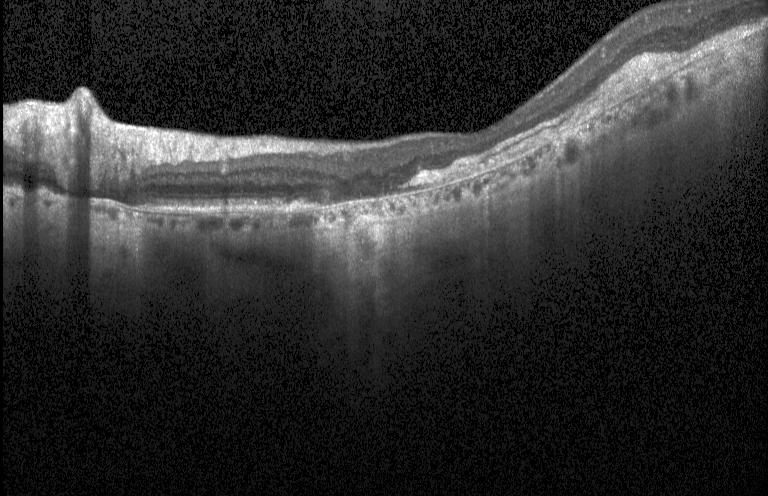 Impression: choroidal neovascularization.